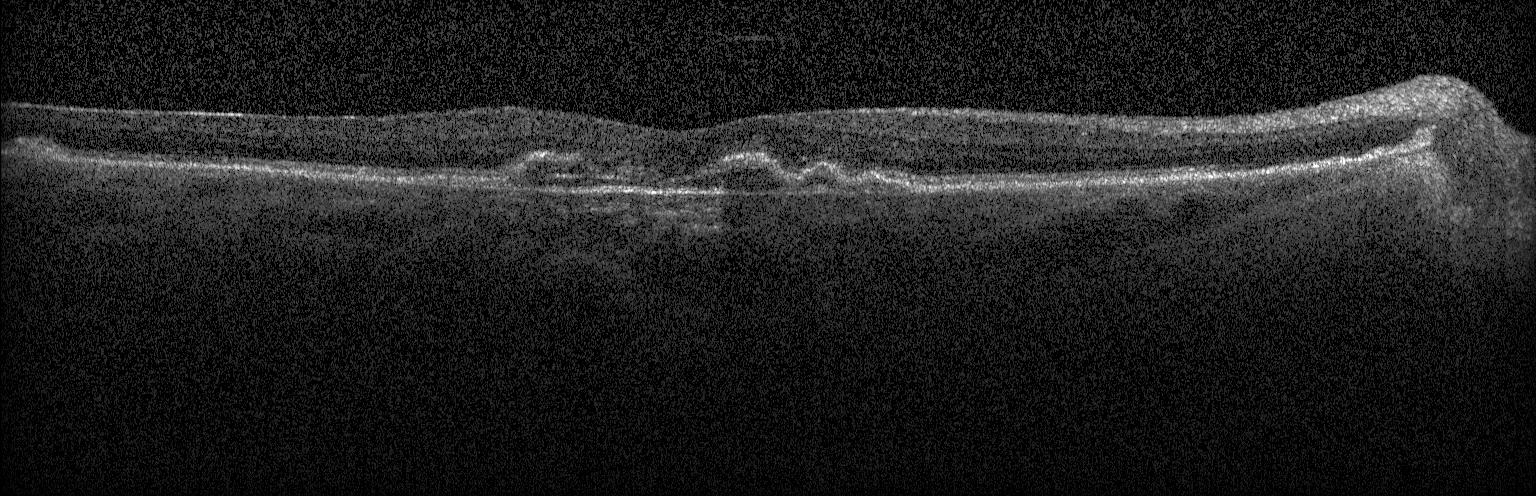 Dx: a choroidal neovascular membrane.